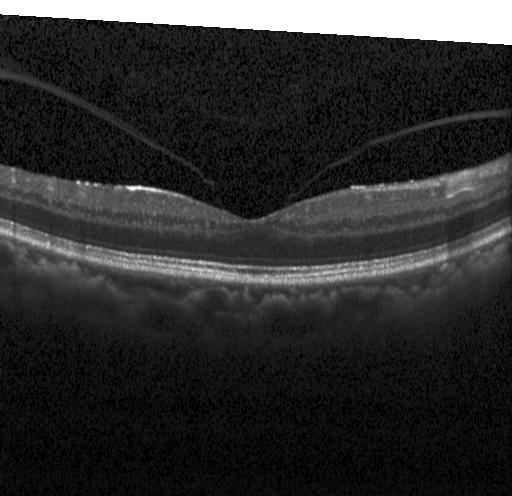 OCT B-scan showing no choroidal neovascularization, no diabetic macular edema, and no drusen.